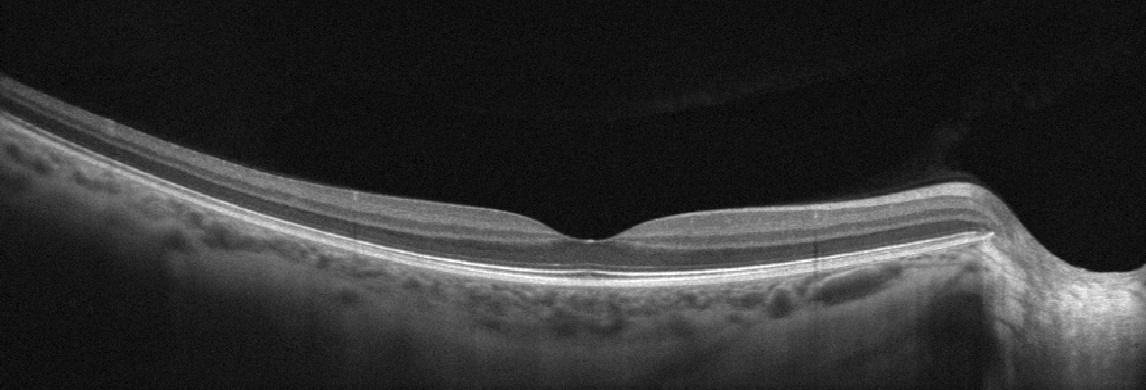
Retinal OCT cross-section; acquired on an Optovue Avanti RTVue XR. Dx: no evidence of AMD, DME, ERM, RAO, RVO, or VID.